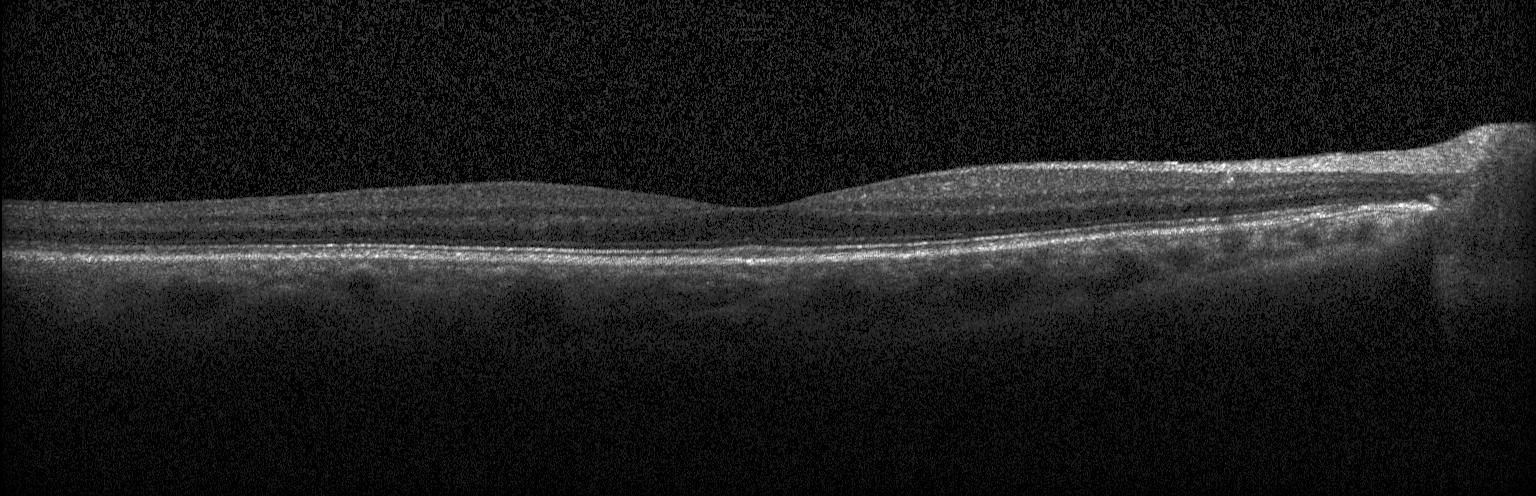

Optical coherence tomography B-scan. Finding: no choroidal neovascularization, no diabetic macular edema, and no drusen.